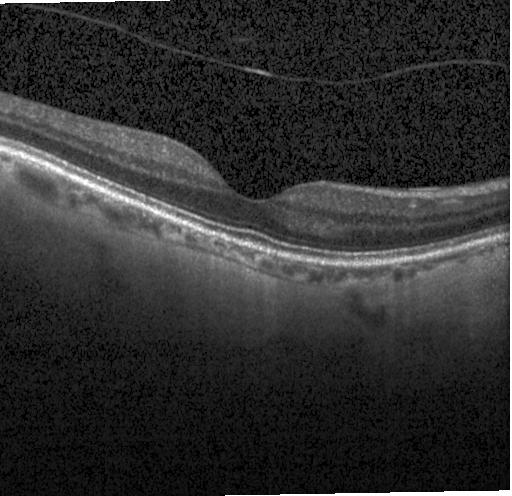
OCT line scan
Finding: no choroidal neovascularization, no diabetic macular edema, and no drusen.